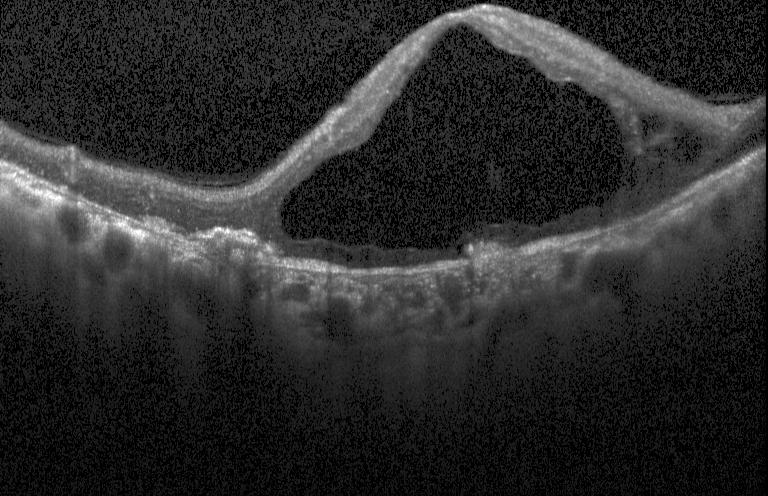 OCT B-scan; fovea-centered — This B-scan demonstrates diabetic macular edema.